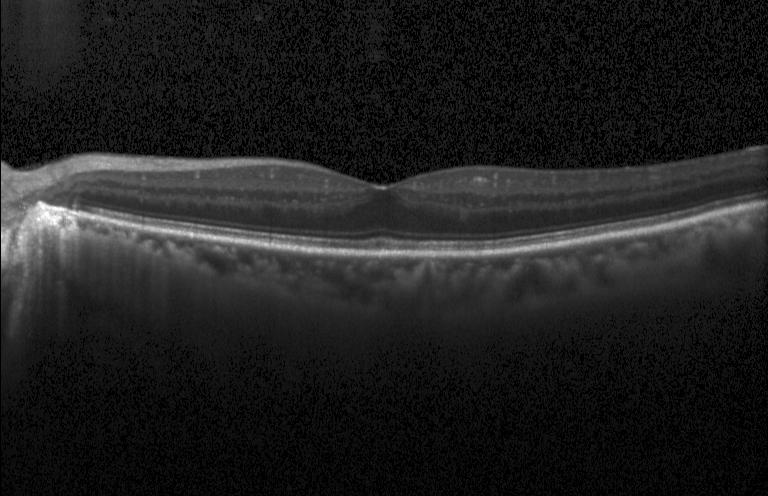

OCT line scan; macular scan
The scan shows no choroidal neovascularization, diabetic macular edema, or drusen.